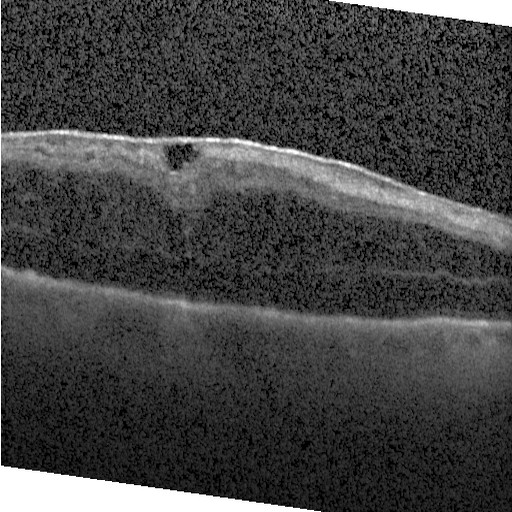 Centered on the fovea · optical coherence tomography scan · spectral-domain OCT.
OCT finding: diabetic macular edema (DME).